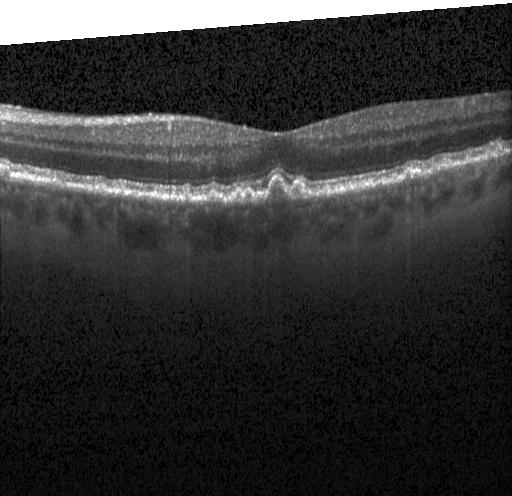 Assessment: sub-RPE drusenoid deposits.